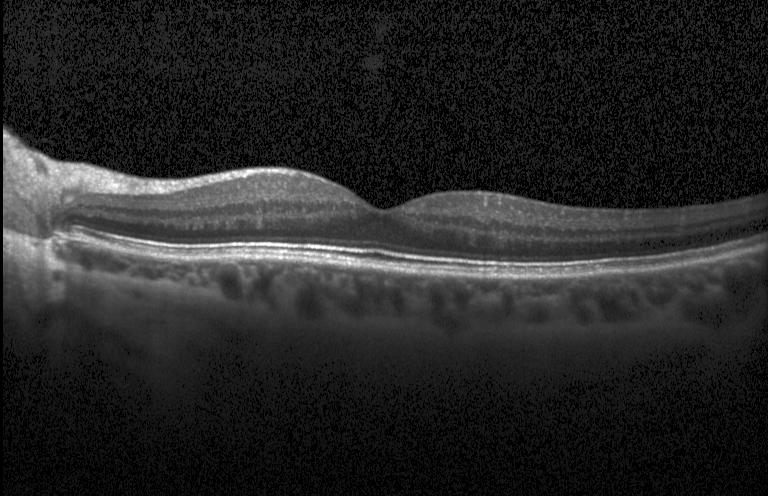 Retinal OCT cross-section — Assessment: no CNV, DME, or drusen.